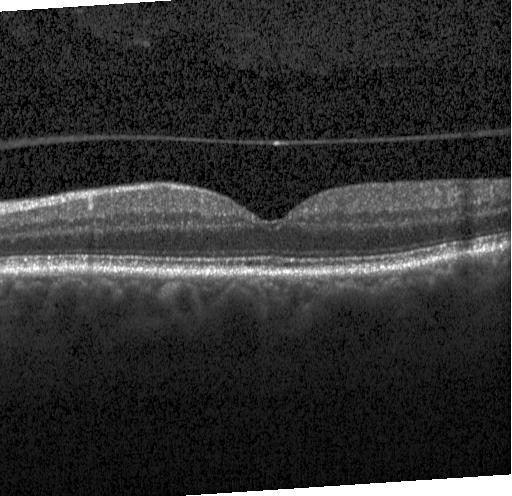

Centered on the fovea. OCT line scan. Spectral-domain OCT. Acquired on a Heidelberg Spectralis. This B-scan demonstrates neither choroidal neovascularization, diabetic macular edema, nor drusen.